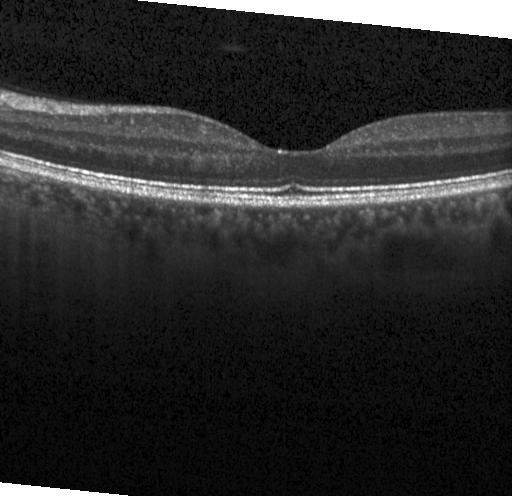

Heidelberg Spectralis. OCT line scan. Macular scan. Spectral-domain OCT — This B-scan demonstrates no choroidal neovascularization, diabetic macular edema, or drusen.